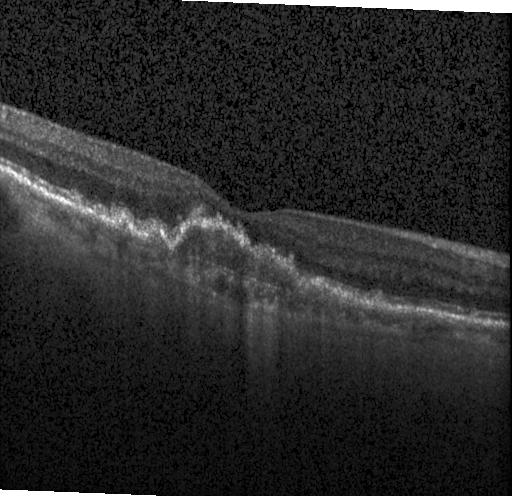 Centered on the fovea, spectral-domain optical coherence tomography, Heidelberg Spectralis, retinal OCT cross-section. Finding: choroidal neovascularization (CNV).